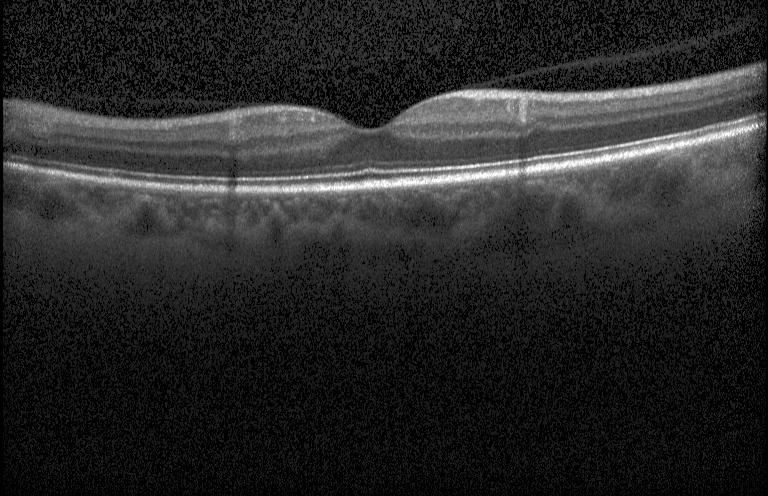

Acquired on a Heidelberg Spectralis · OCT B-scan · fovea-centered
Diagnosis: neither choroidal neovascularization, diabetic macular edema, nor drusen.